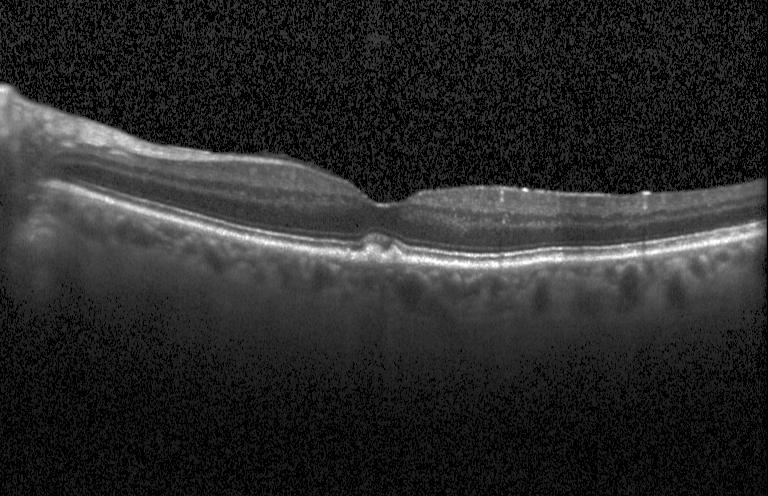
Finding: sub-RPE drusenoid deposits.